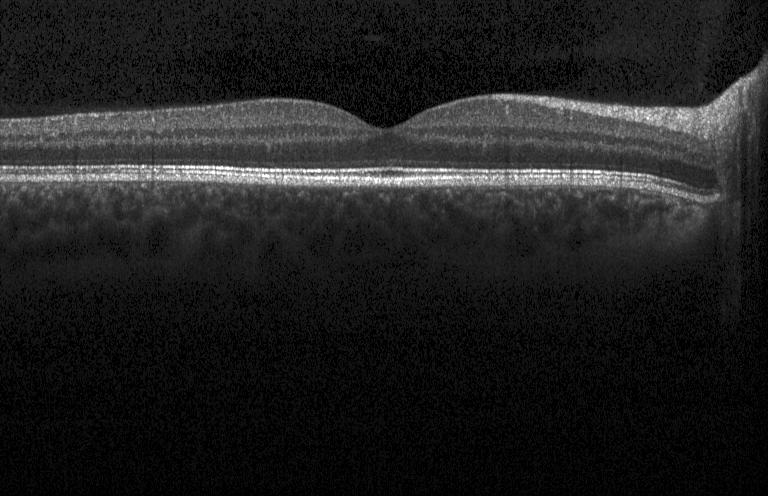

This B-scan demonstrates neither choroidal neovascularization, diabetic macular edema, nor drusen.